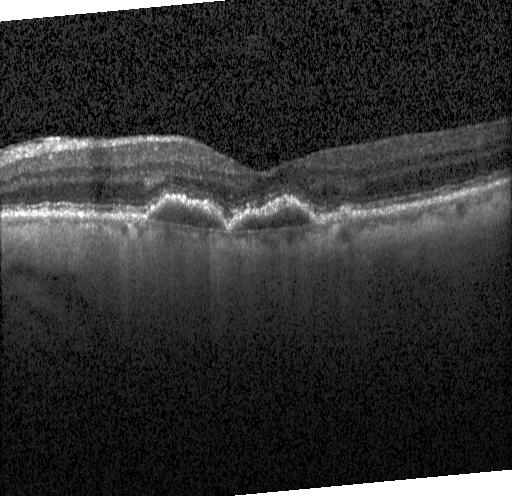 Optical coherence tomography B-scan. Through the macula. CNV.